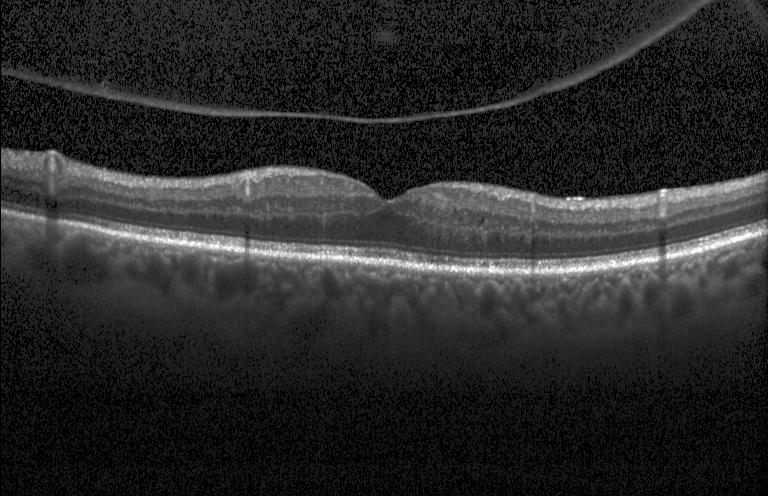
Macular OCT demonstrating neither CNV, DME, nor drusen.